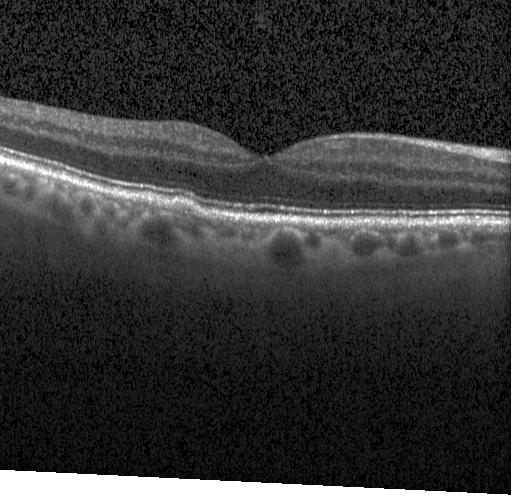

OCT scan showing sub-RPE drusenoid deposits.